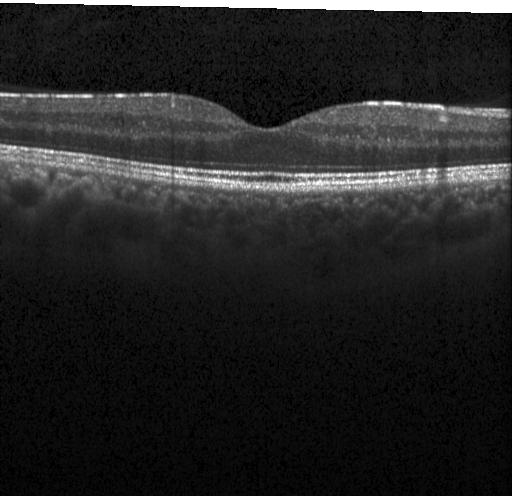

SD-OCT; OCT B-scan.
Finding: neither choroidal neovascularization, diabetic macular edema, nor drusen.